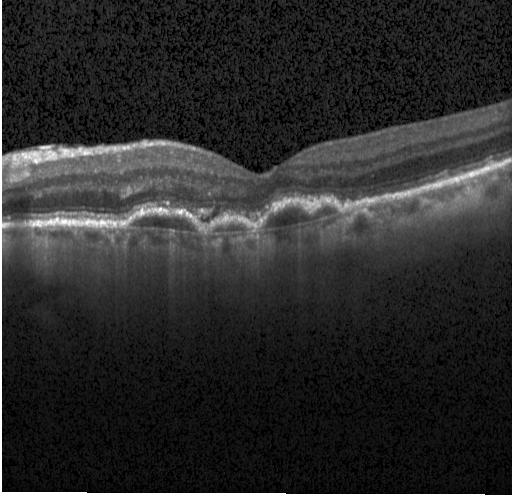
Finding: CNV.